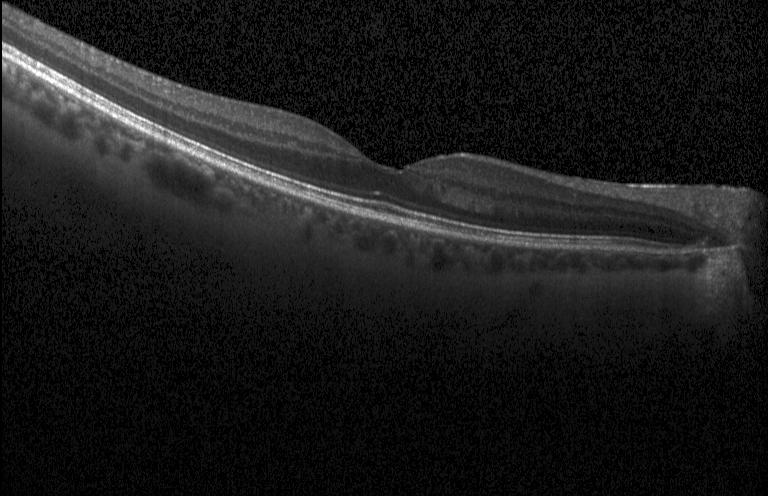
Finding: no choroidal neovascularization, no diabetic macular edema, and no drusen.